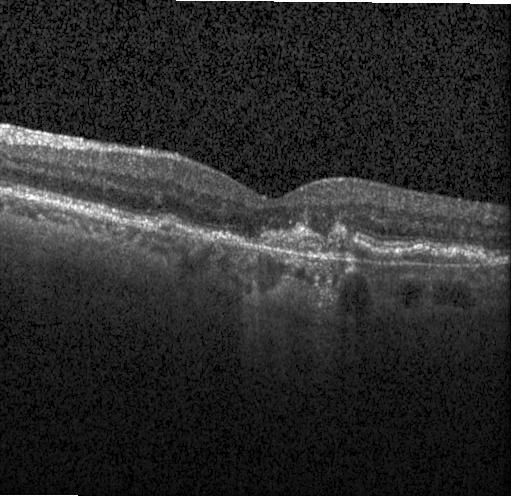

Retinal OCT B-scan · fovea-centered · spectral-domain OCT · Heidelberg Spectralis OCT system. OCT finding: CNV.